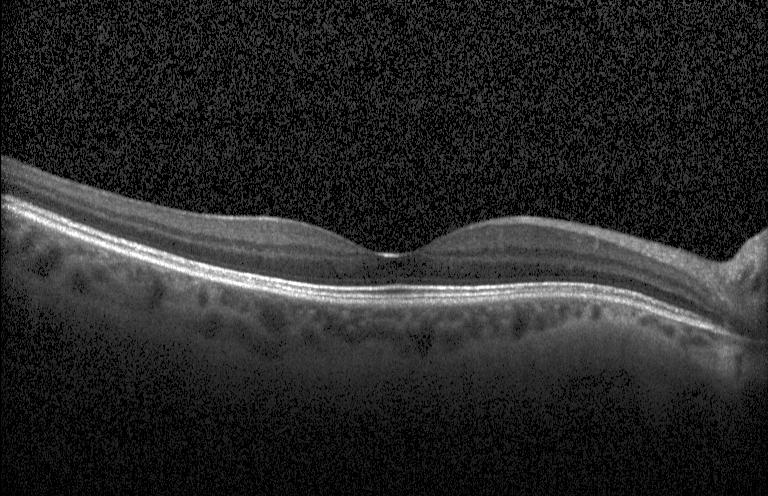
Spectral-domain OCT B-scan: no evidence of choroidal neovascularization, diabetic macular edema, or drusen.